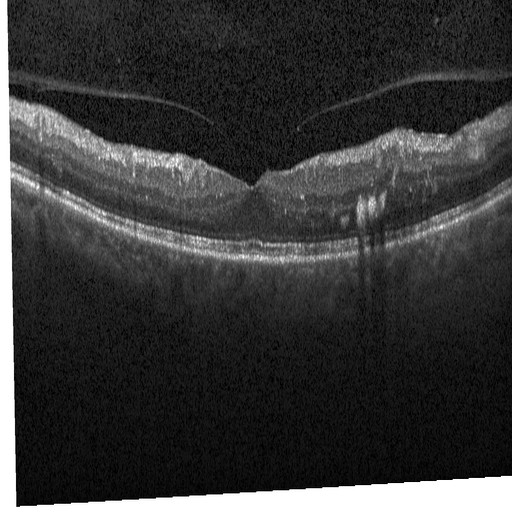

OCT B-scan, spectral-domain OCT
OCT finding: diabetic macular edema (DME).